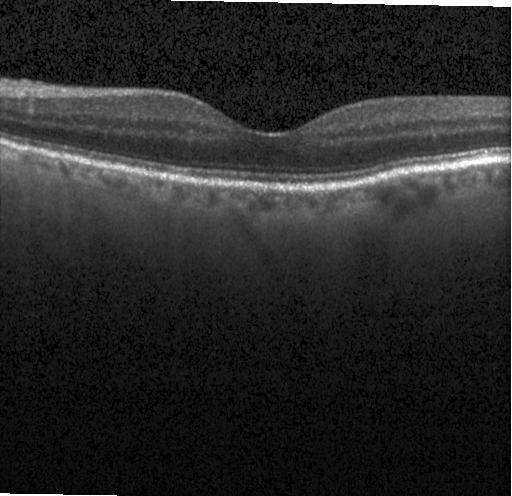 Retinal OCT cross-section · SD-OCT · instrument: Heidelberg Spectralis
Impression: no choroidal neovascularization, no diabetic macular edema, and no drusen.